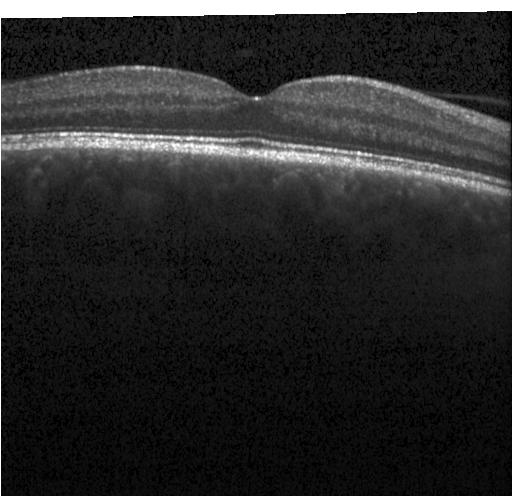 Optical coherence tomography B-scan. Heidelberg Spectralis
Assessment: no choroidal neovascularization, diabetic macular edema, or drusen.